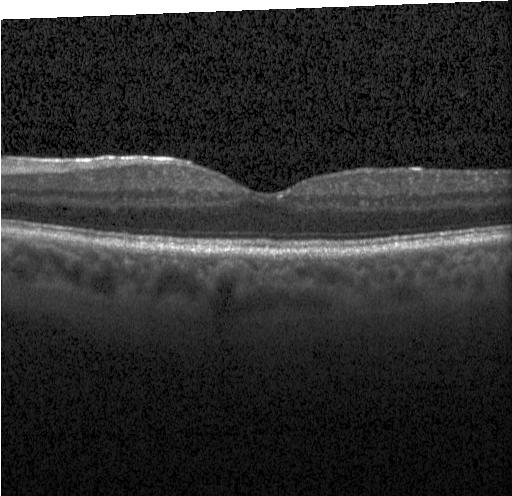
Diagnosis: neither choroidal neovascularization, diabetic macular edema, nor drusen.